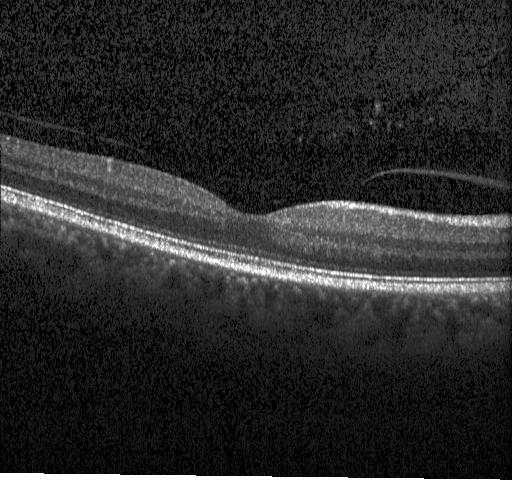
Impression: neither choroidal neovascularization, diabetic macular edema, nor drusen.